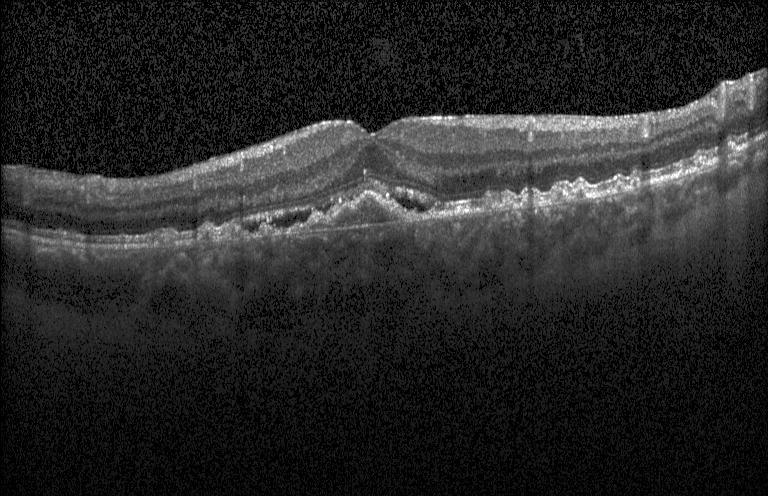

Spectral-domain OCT B-scan: a choroidal neovascular membrane.